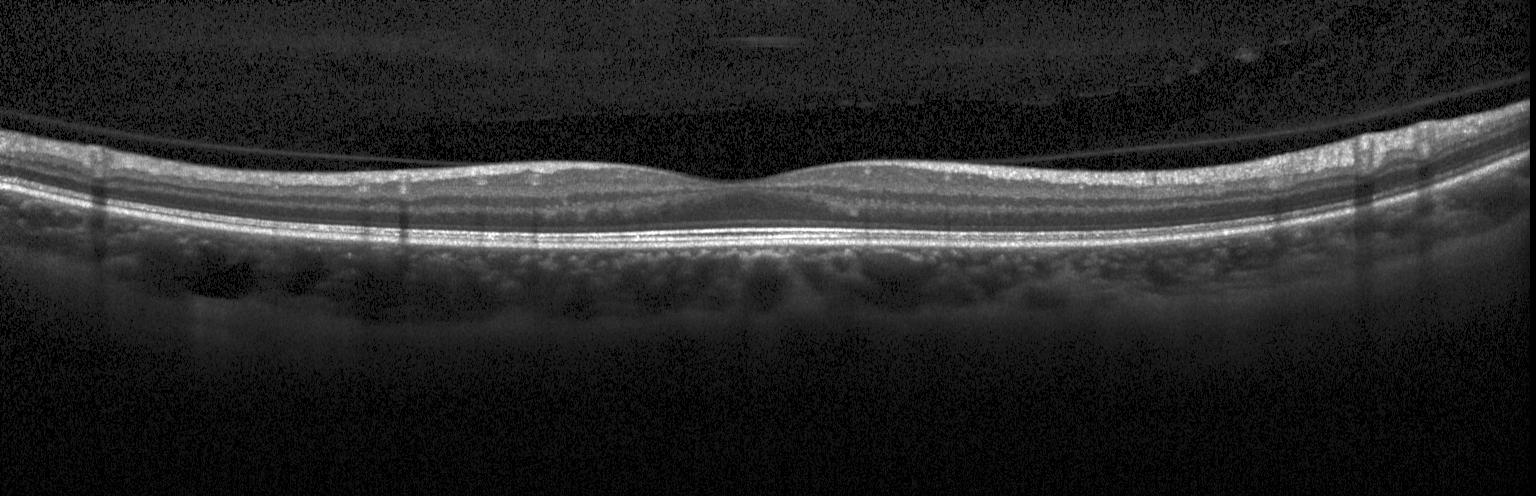 Fovea-centered. Acquired on a Heidelberg Spectralis. OCT B-scan. Assessment: no choroidal neovascularization, diabetic macular edema, or drusen.